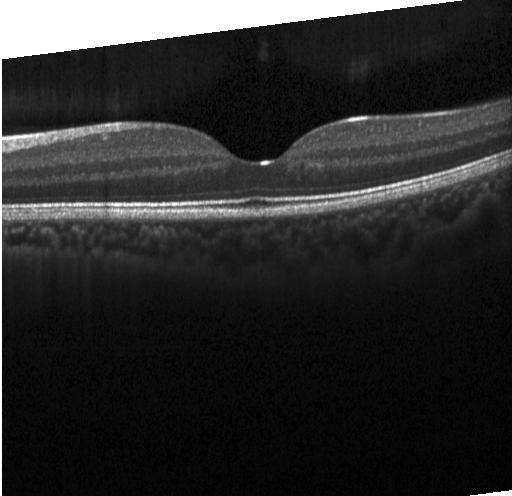 Spectral-domain OCT · acquired on a Heidelberg Spectralis · fovea-centered · OCT B-scan — The scan shows no choroidal neovascularization, diabetic macular edema, or drusen.